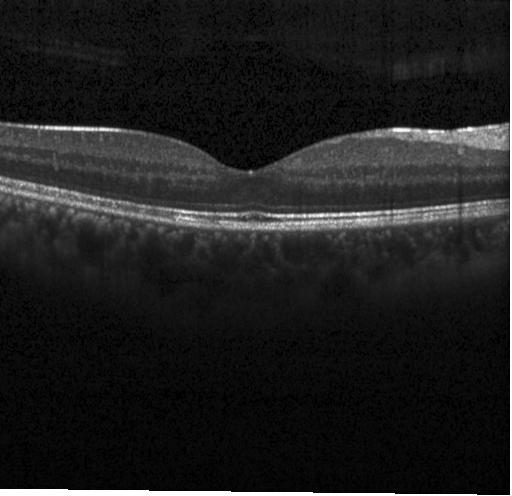
Diagnosis: no choroidal neovascularization, diabetic macular edema, or drusen.